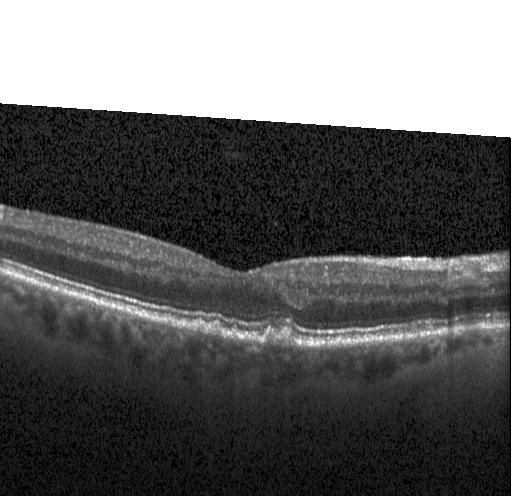
Acquired on a Heidelberg Spectralis · spectral-domain optical coherence tomography · retinal OCT B-scan. Impression: drusen.